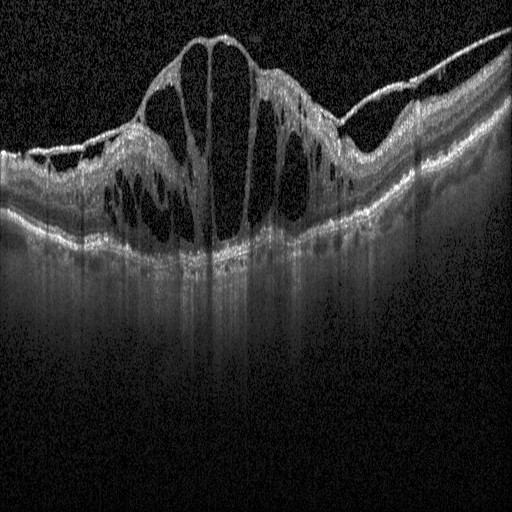
OCT line scan, through the macula
Assessment: diabetic macular edema (DME).